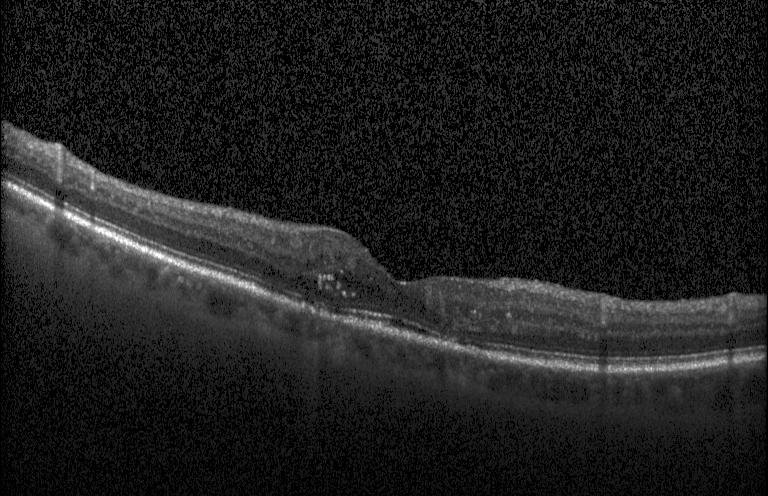
Spectral-domain OCT; optical coherence tomography scan.
Finding: diabetic macular edema (DME).